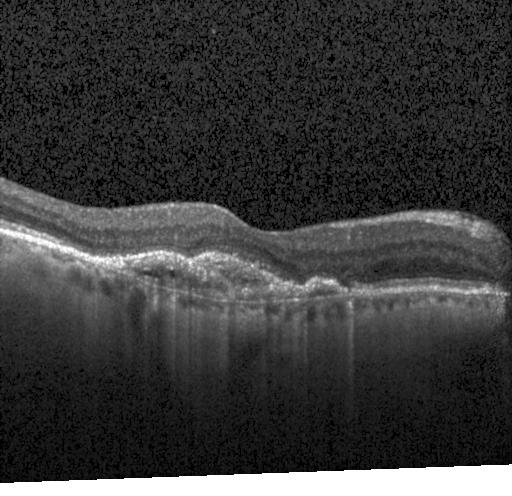
Dx: a choroidal neovascular membrane.